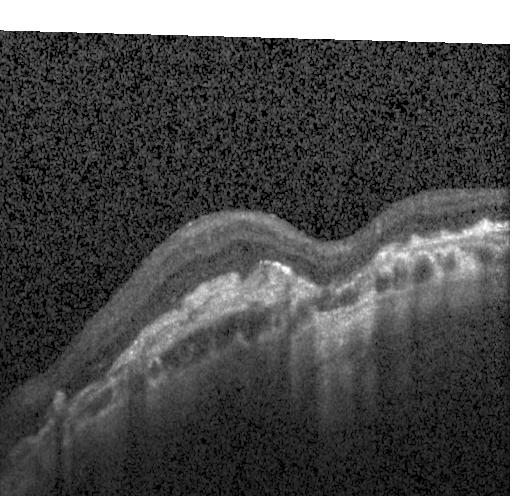

OCT scan showing a choroidal neovascular membrane.